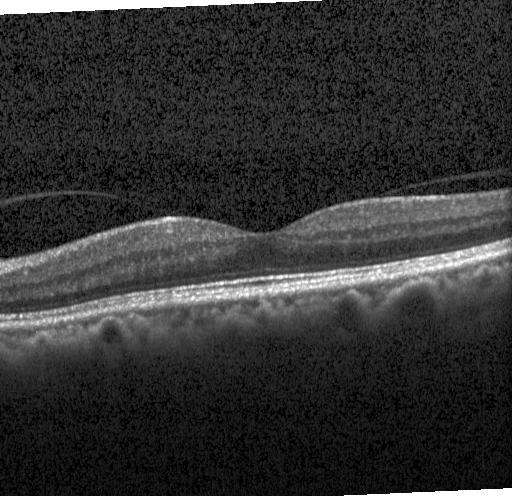

Retinal OCT cross-section, macular scan.
This B-scan demonstrates no CNV, DME, or drusen.